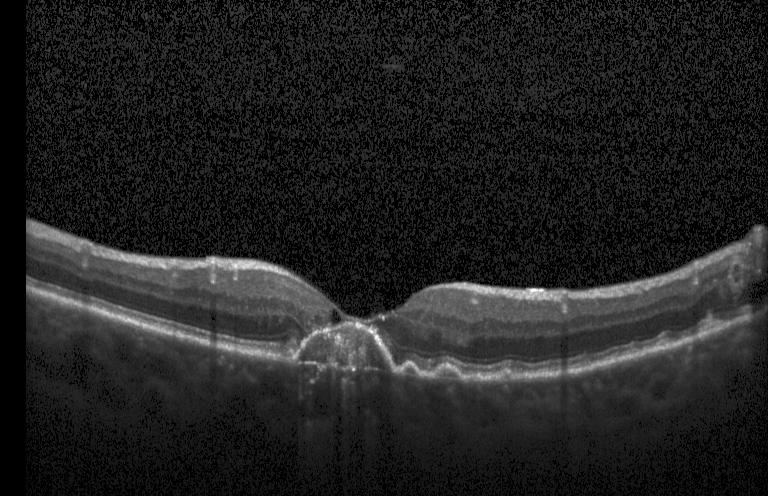 Retinal OCT B-scan. Horizontal scan through the fovea.
This B-scan demonstrates a choroidal neovascular membrane.